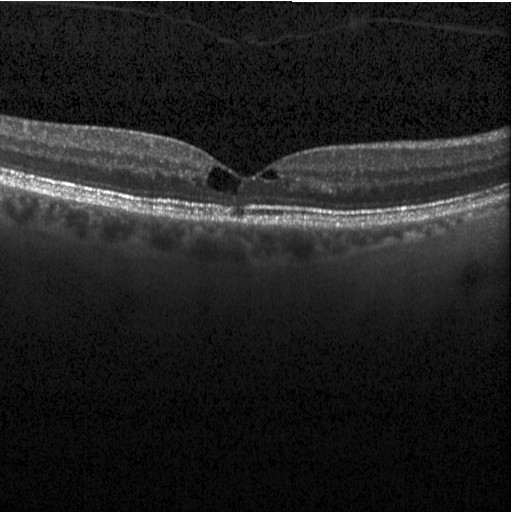 Optical coherence tomography B-scan · Heidelberg Spectralis
Diagnosis: diabetic macular edema (DME).